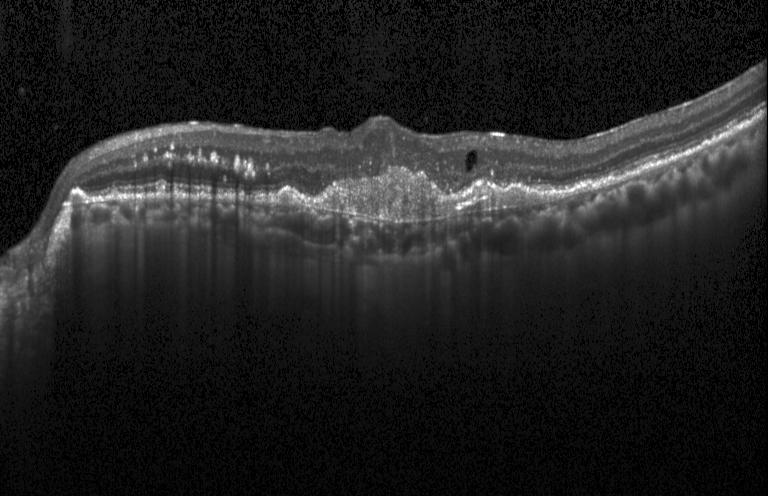

SD-OCT. Retinal OCT B-scan. Finding: CNV.